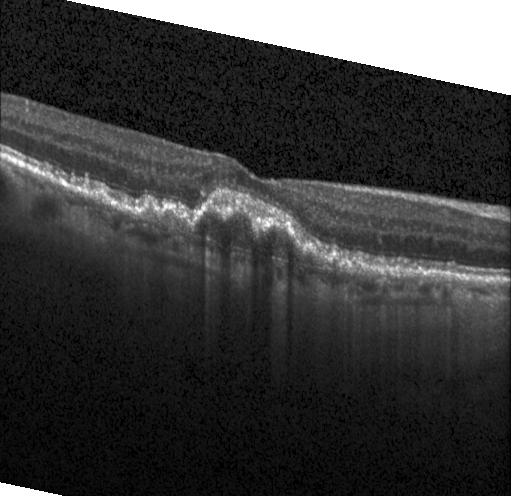

OCT finding: a choroidal neovascular membrane.